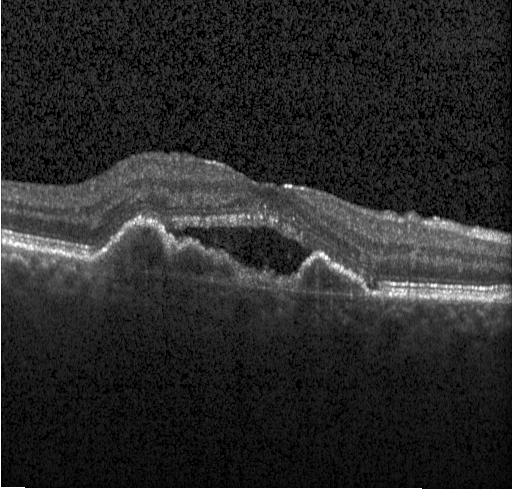
Assessment: choroidal neovascularization.